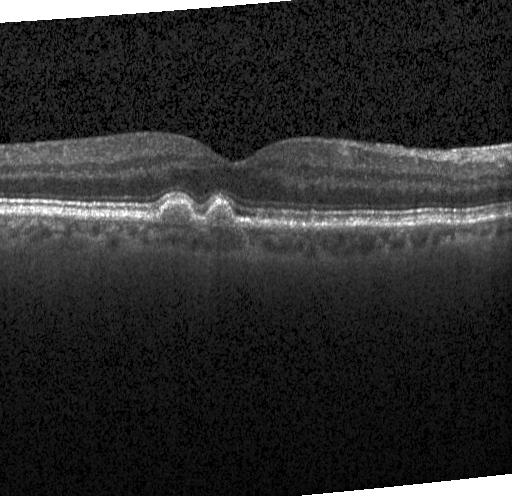 Assessment: multiple drusen.